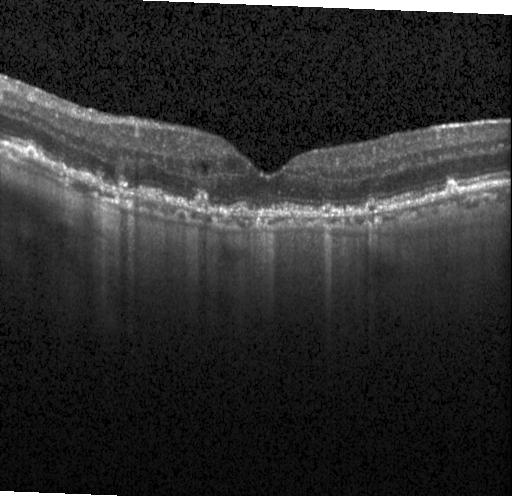

Dx: a choroidal neovascular membrane.